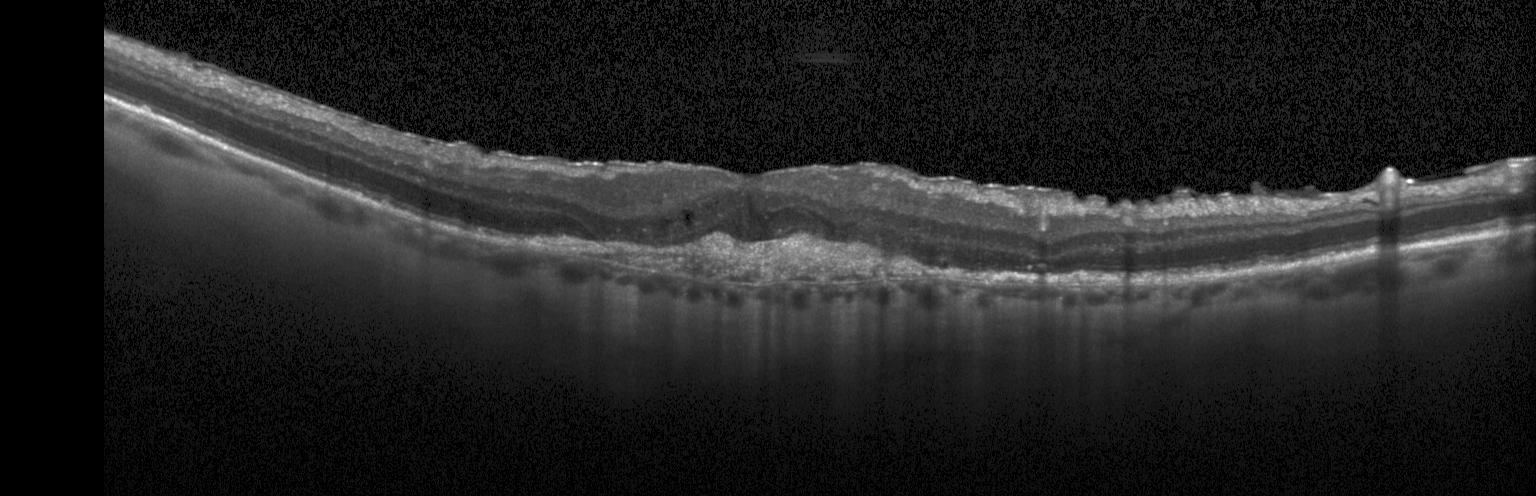 Through the macula. Acquired on a Heidelberg Spectralis. SD-OCT. OCT line scan — This B-scan demonstrates a choroidal neovascular membrane.